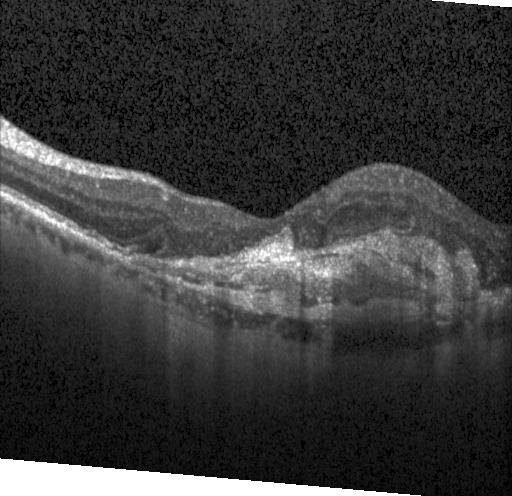
Optical coherence tomography B-scan. Finding: choroidal neovascularization (CNV).